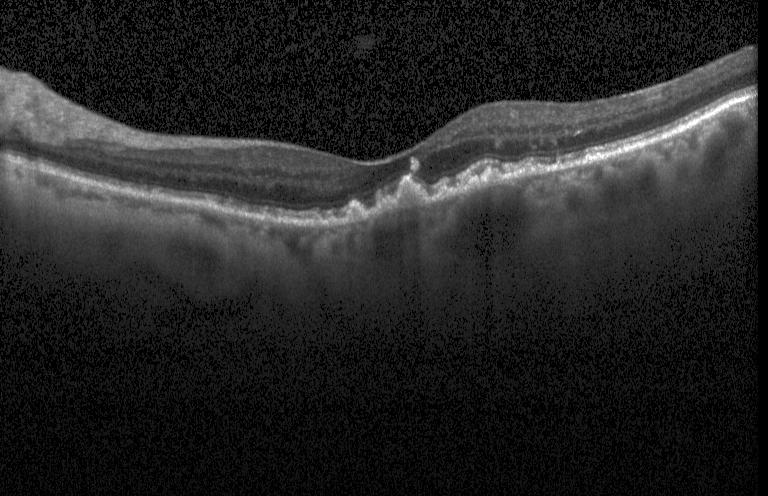

Dx: drusen.